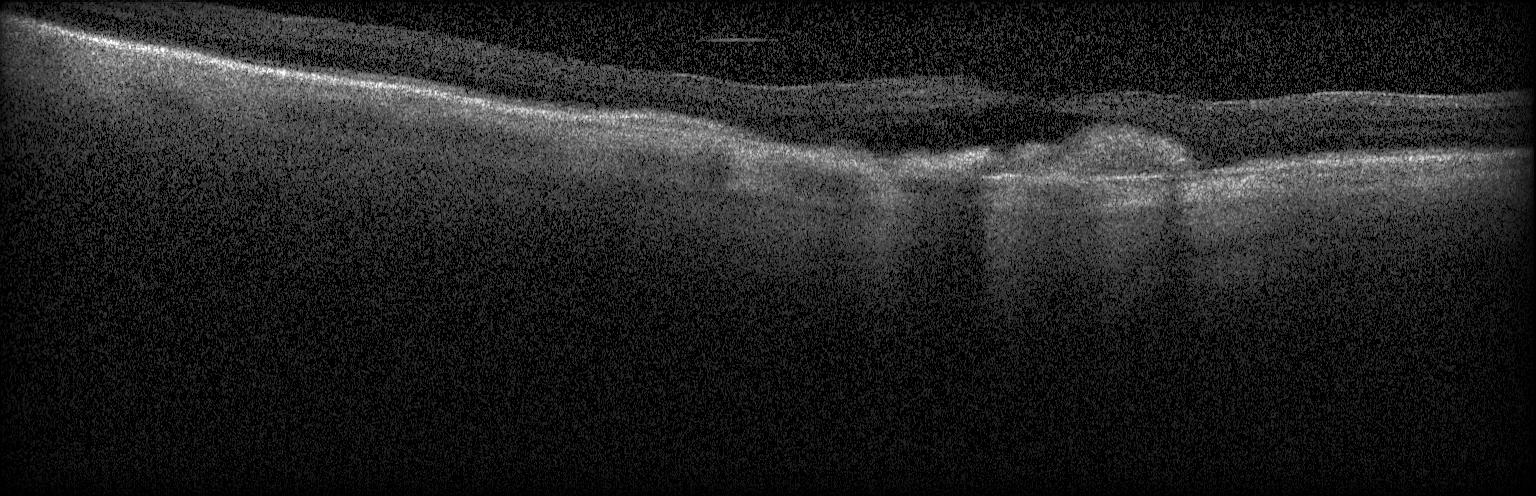 Diagnosis: a choroidal neovascular membrane.